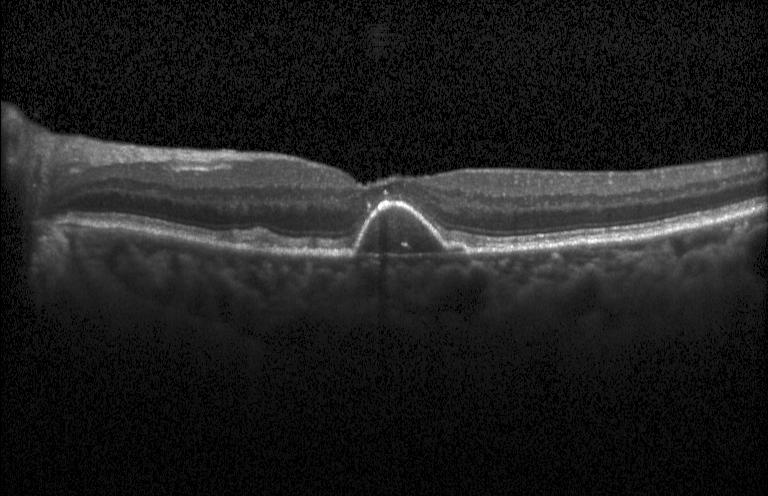 Dx: a choroidal neovascular membrane.